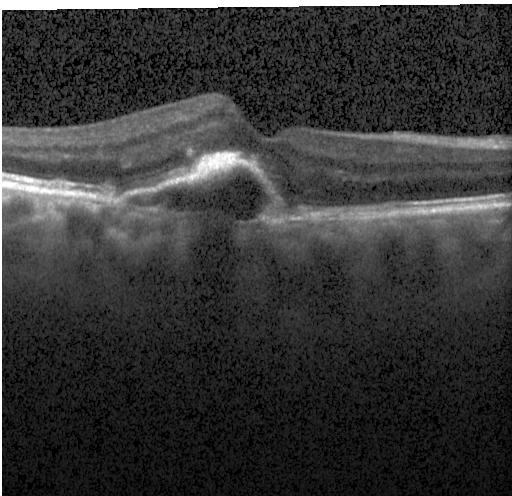
Retinal OCT B-scan
Macular OCT: choroidal neovascularization.